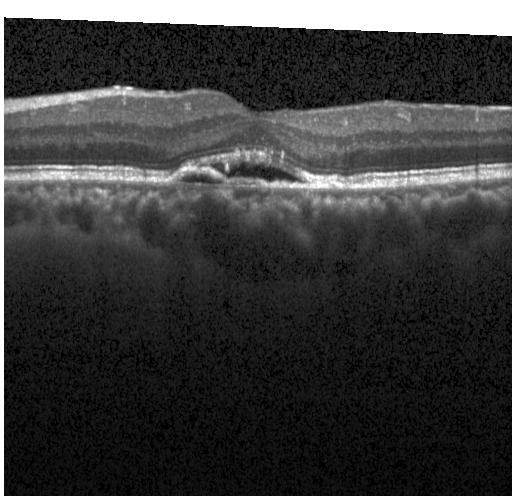
Fovea-centered · acquired on a Heidelberg Spectralis · spectral-domain optical coherence tomography · retinal OCT cross-section.
Finding: choroidal neovascularization.